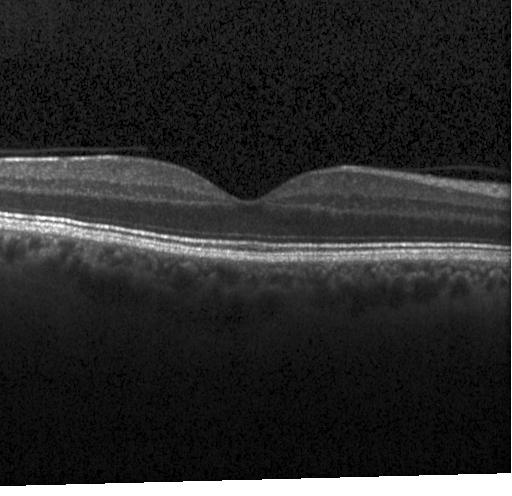 OCT line scan
No choroidal neovascularization, no diabetic macular edema, and no drusen.